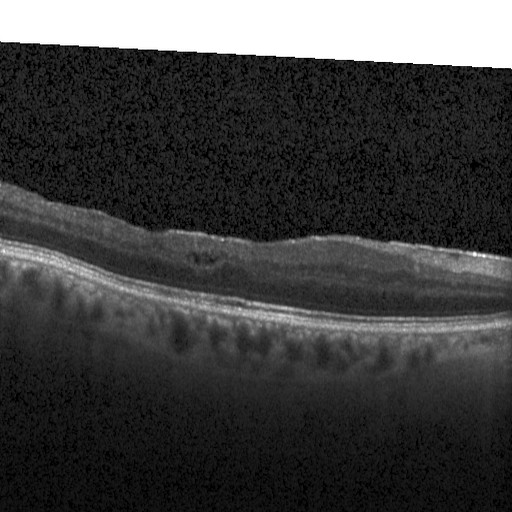
Macular OCT demonstrating diabetic macular edema.